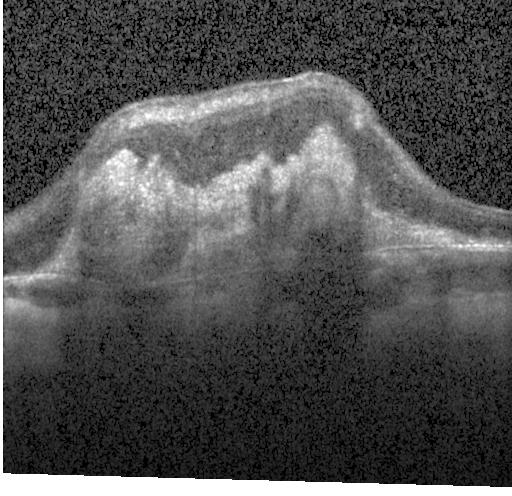
Retinal OCT cross-section. Heidelberg Spectralis OCT system. Through the macula.
Diagnosis: a choroidal neovascular membrane.